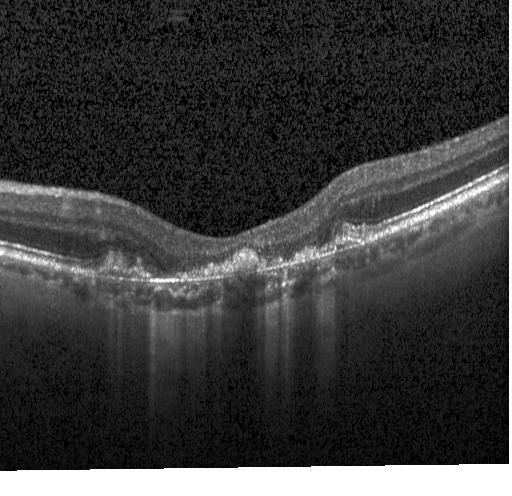 OCT B-scan showing CNV.